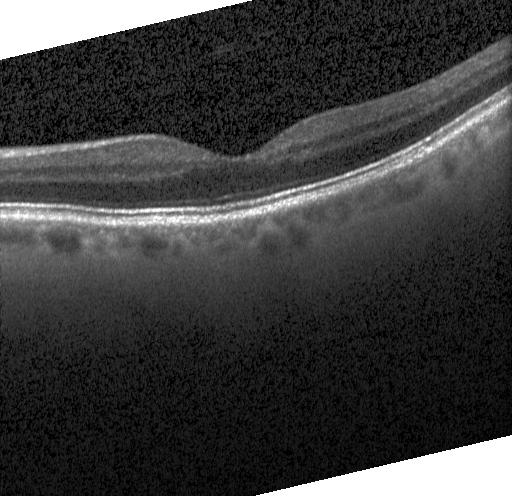

Impression: no choroidal neovascularization, no diabetic macular edema, and no drusen.